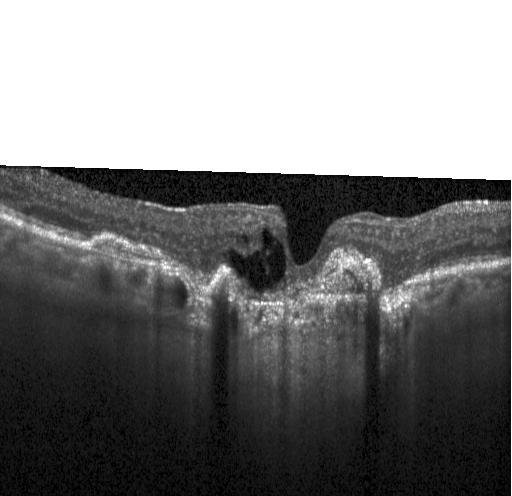
OCT scan showing choroidal neovascularization (CNV).